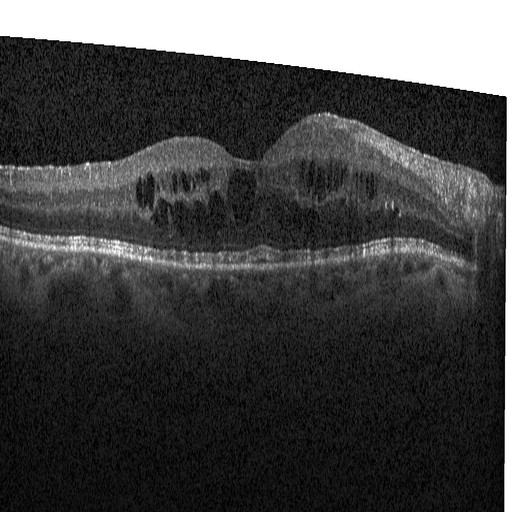
Macular scan, spectral-domain OCT, acquired on a Heidelberg Spectralis, optical coherence tomography B-scan. Impression: diabetic macular edema.